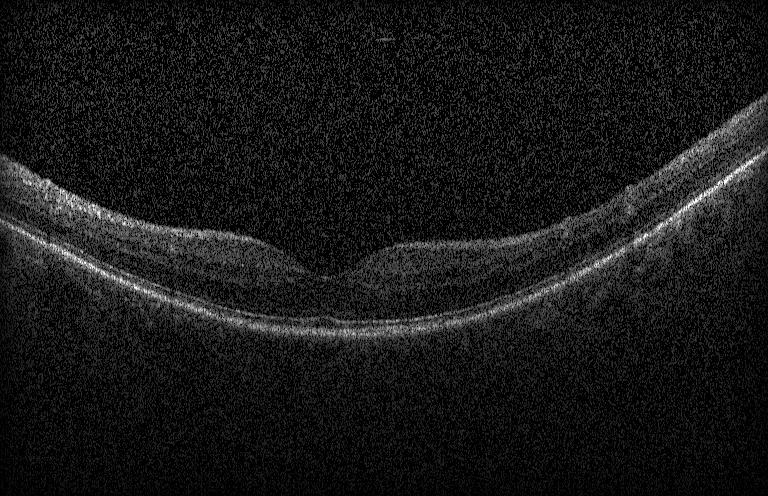

Macular OCT demonstrating neither CNV, DME, nor drusen.